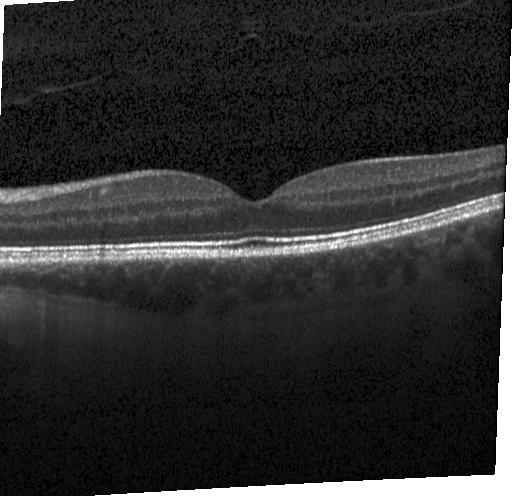 Acquired on a Heidelberg Spectralis; optical coherence tomography scan; spectral-domain OCT
Impression: neither CNV, DME, nor drusen.